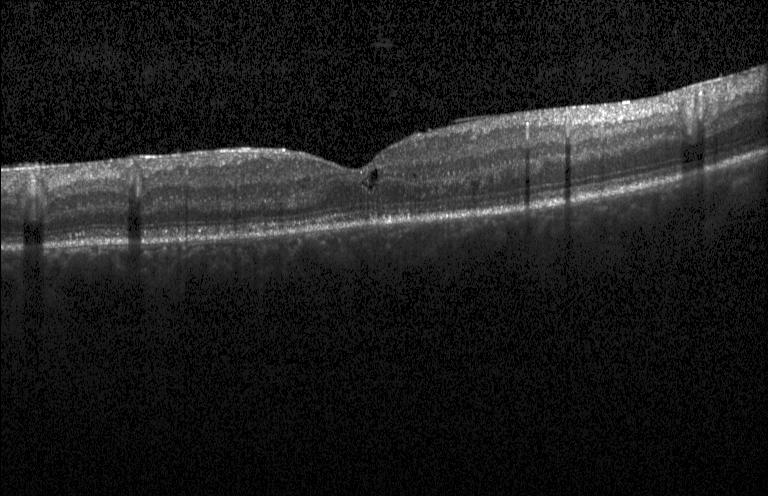
Retinal OCT B-scan. Diabetic macular edema (DME).